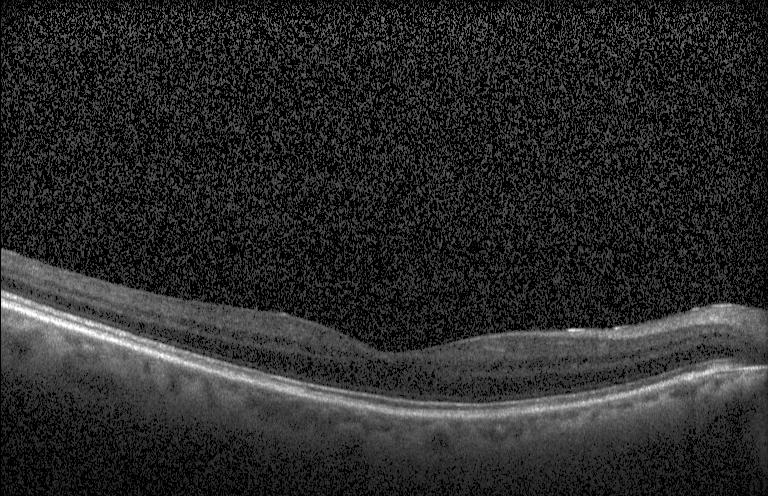
Heidelberg Spectralis OCT system, retinal OCT B-scan, spectral-domain optical coherence tomography — The scan shows neither choroidal neovascularization, diabetic macular edema, nor drusen.